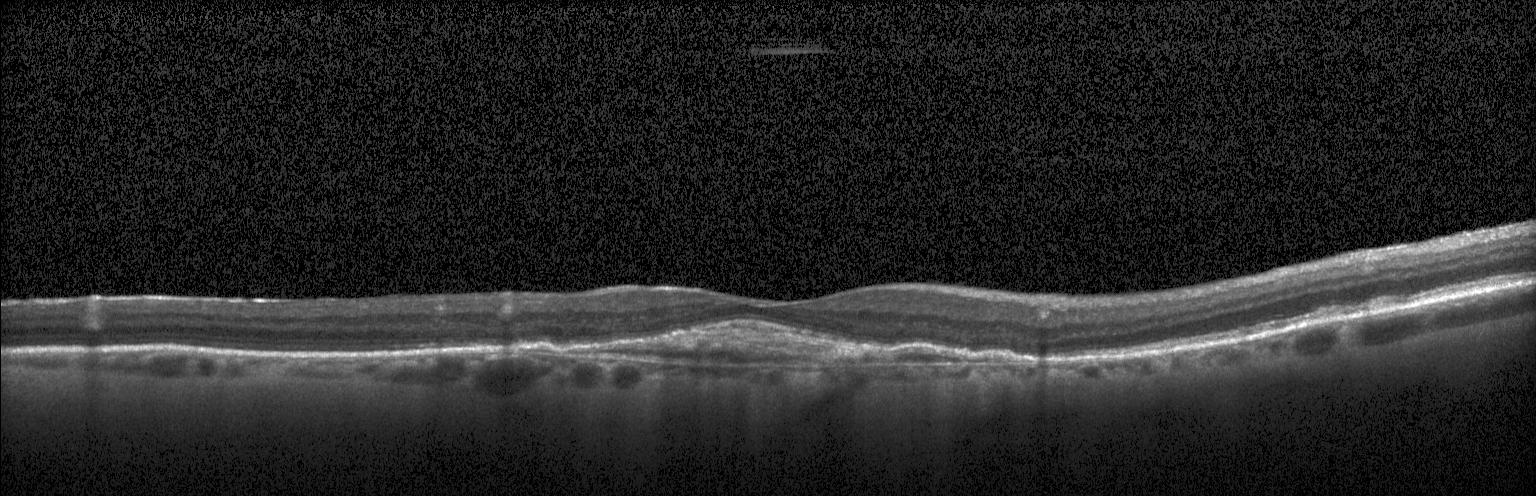
Heidelberg Spectralis OCT system, SD-OCT, optical coherence tomography scan
Diagnosis: CNV.